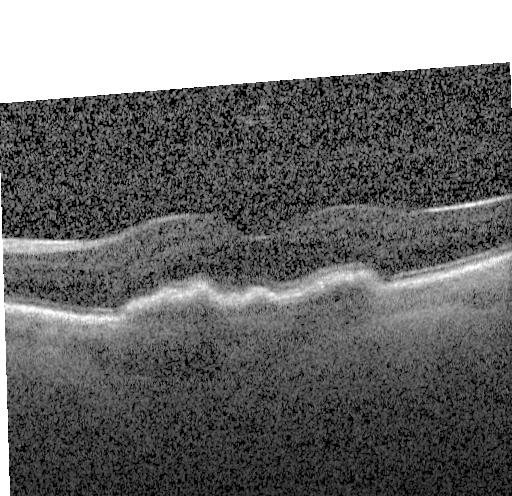 Horizontal scan through the fovea; retinal OCT cross-section — Finding: a choroidal neovascular membrane.